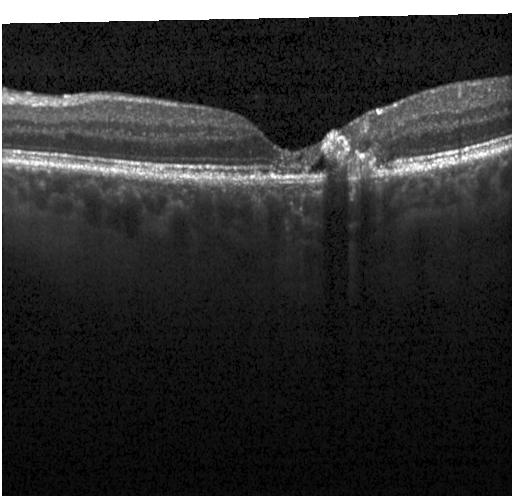

Heidelberg Spectralis OCT system, OCT line scan, horizontal scan through the fovea, spectral-domain optical coherence tomography — OCT finding: a choroidal neovascular membrane.